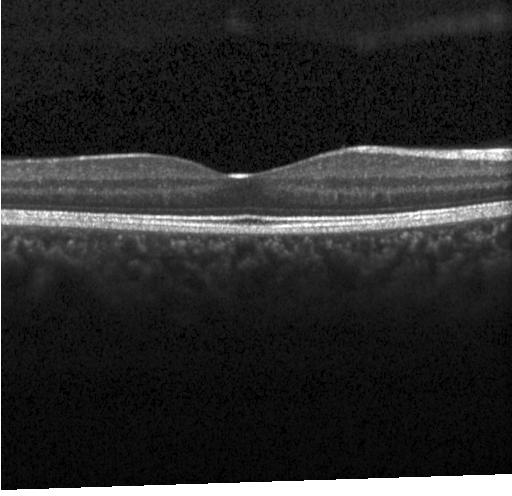 Impression: no choroidal neovascularization, diabetic macular edema, or drusen.